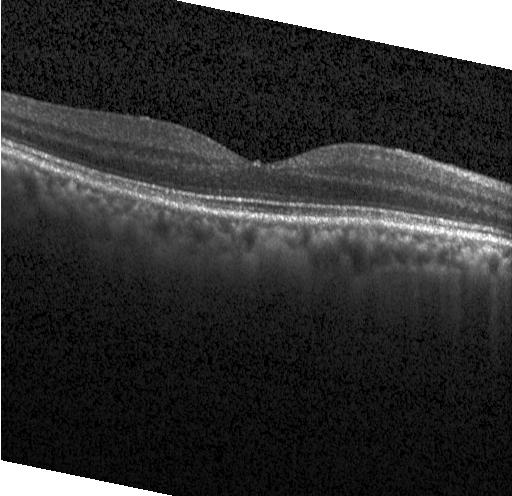
Retinal OCT cross-section
Assessment: no evidence of choroidal neovascularization, diabetic macular edema, or drusen.